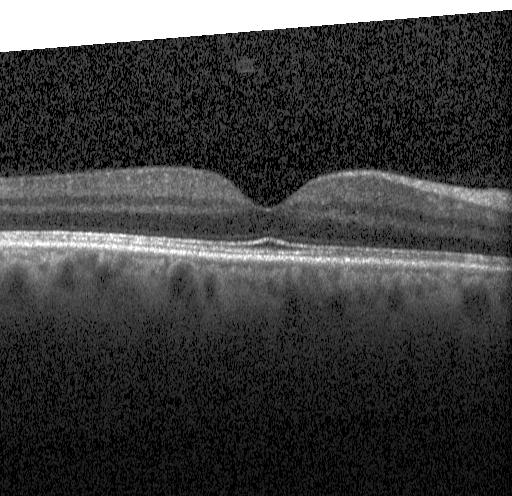

Centered on the fovea, retinal OCT cross-section — Finding: no choroidal neovascularization, no diabetic macular edema, and no drusen.